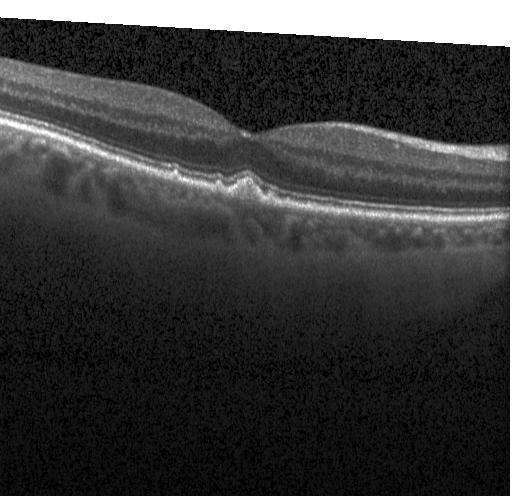 Macular OCT demonstrating multiple drusen.